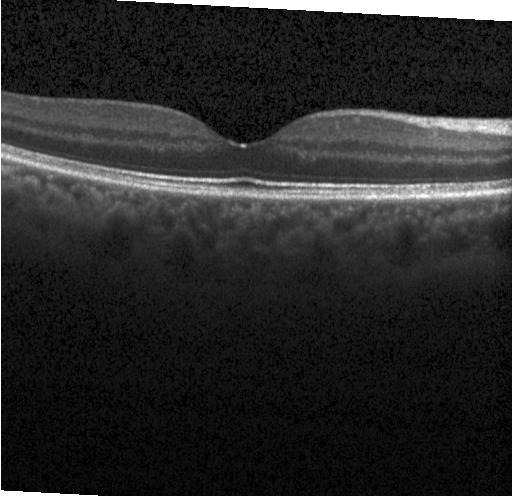 Assessment: no choroidal neovascularization, no diabetic macular edema, and no drusen.